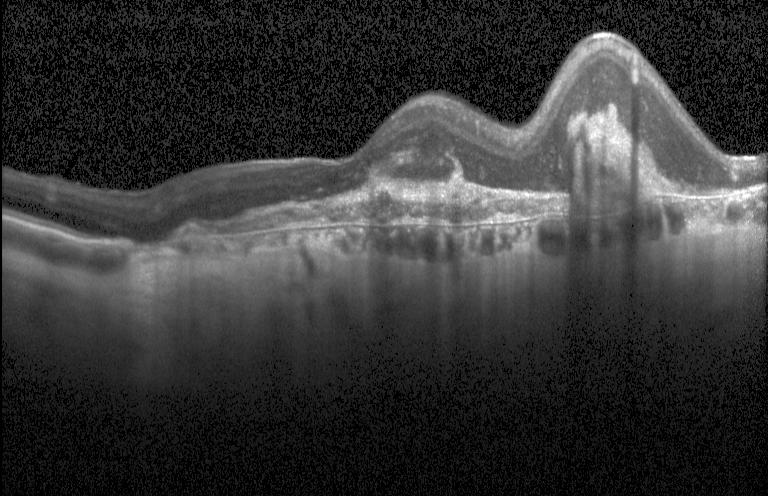
Retinal OCT cross-section showing choroidal neovascularization.